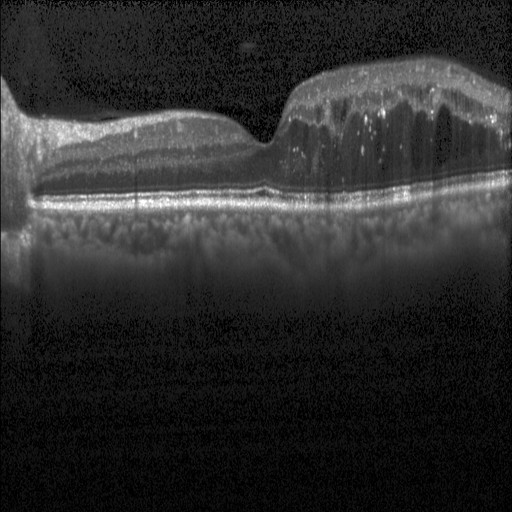
Macular OCT demonstrating diabetic macular edema.